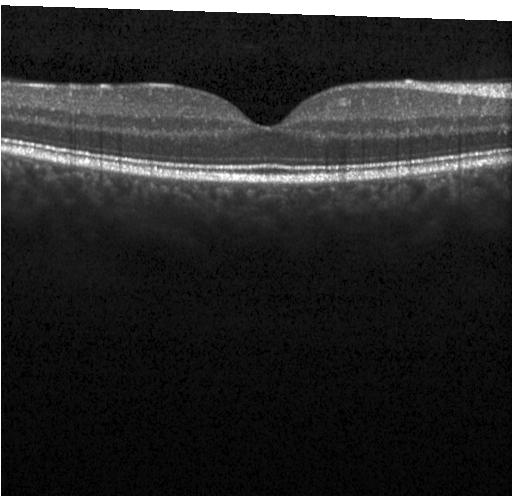

Retinal OCT cross-section; instrument: Heidelberg Spectralis; through the macula. This B-scan demonstrates neither choroidal neovascularization, diabetic macular edema, nor drusen.